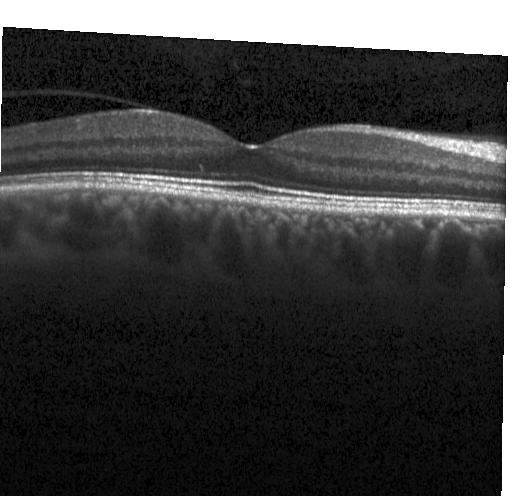
Spectral-domain OCT; acquired on a Heidelberg Spectralis; retinal OCT B-scan; horizontal scan through the fovea. Macular OCT: no choroidal neovascularization, no diabetic macular edema, and no drusen.